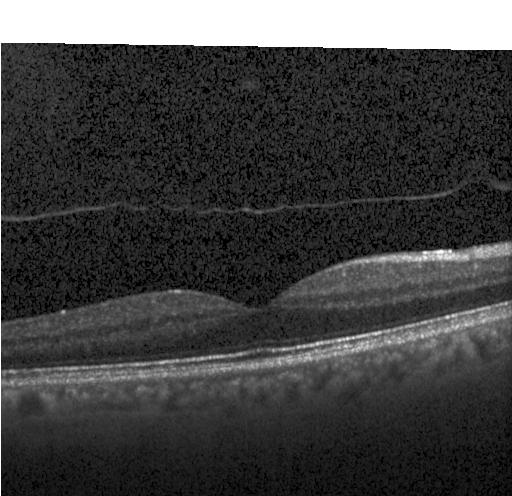

The scan shows no CNV, no DME, and no drusen.